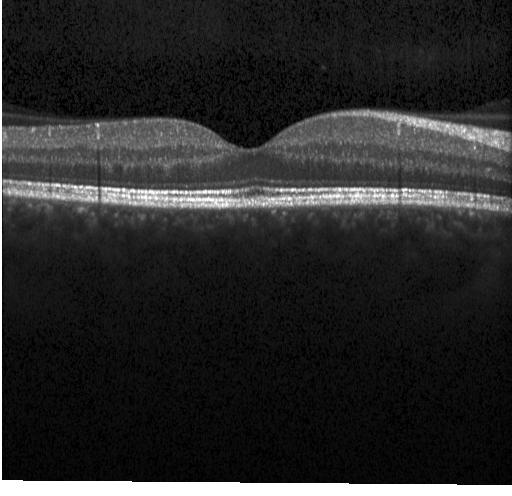
OCT line scan, acquired on a Heidelberg Spectralis, horizontal scan through the fovea — Diagnosis: no choroidal neovascularization, diabetic macular edema, or drusen.